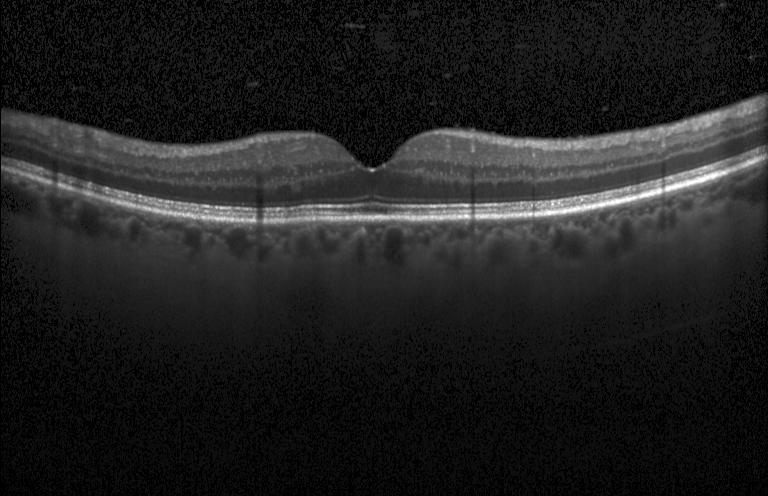
Impression: no evidence of CNV, DME, or drusen.